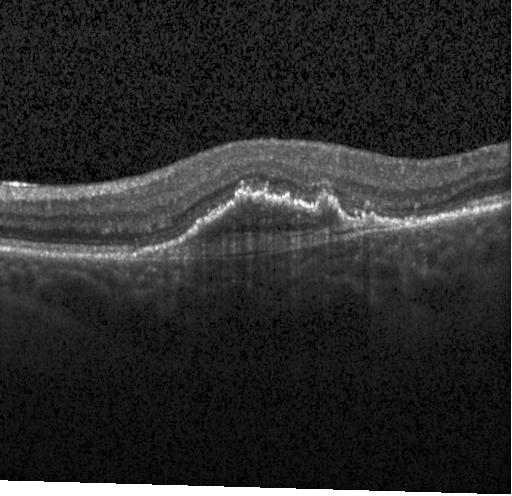
Impression: choroidal neovascularization.